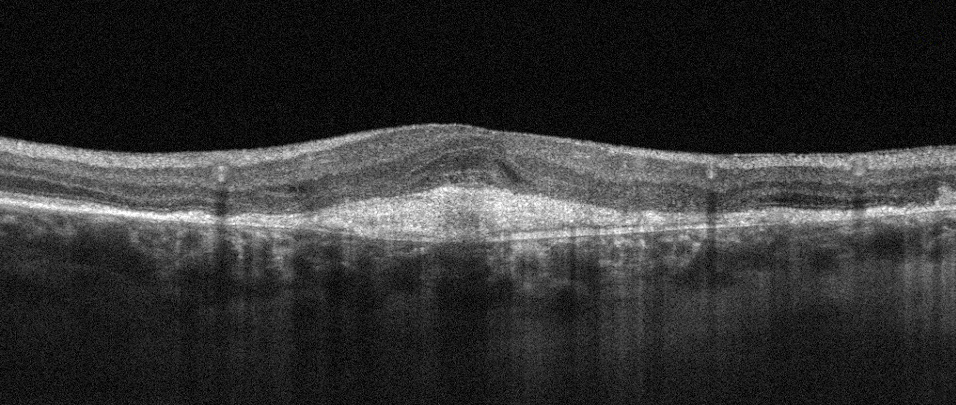

Assessment: AMD.